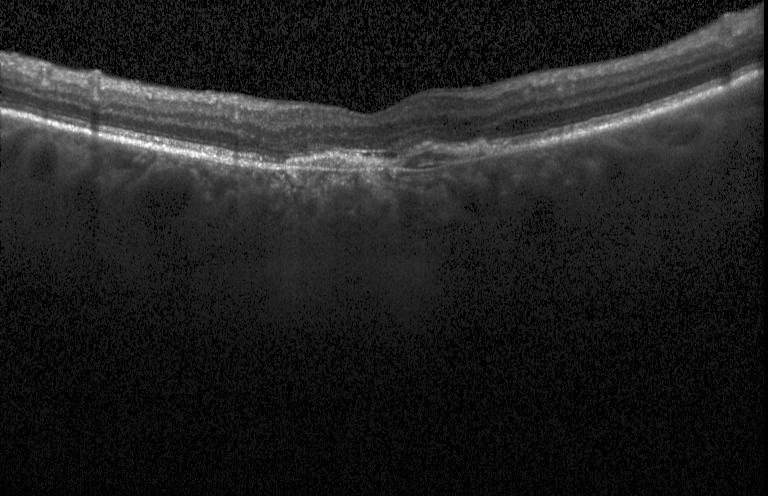 Macular OCT: choroidal neovascularization.